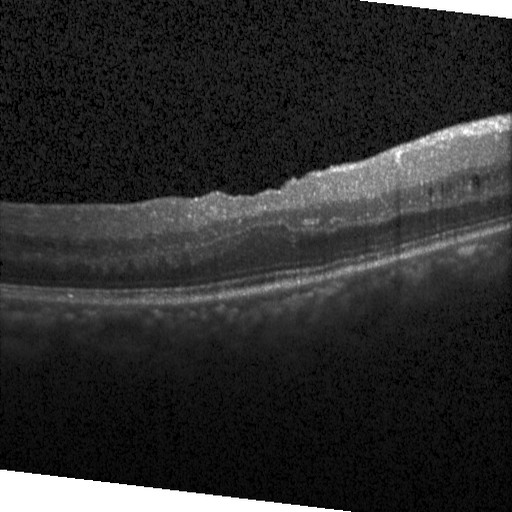 OCT line scan.
Finding: diabetic macular edema.